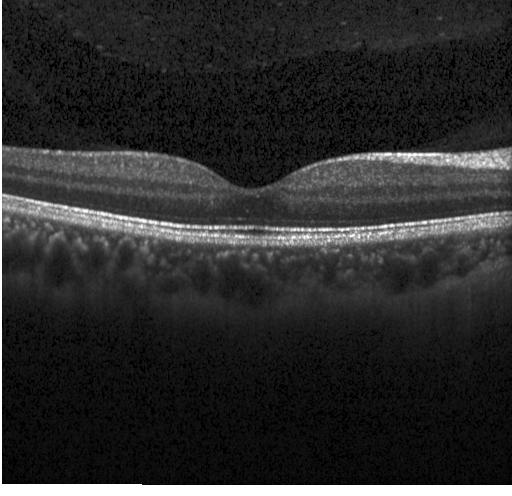
Retinal OCT cross-section. Heidelberg Spectralis. SD-OCT
The scan shows no evidence of CNV, DME, or drusen.